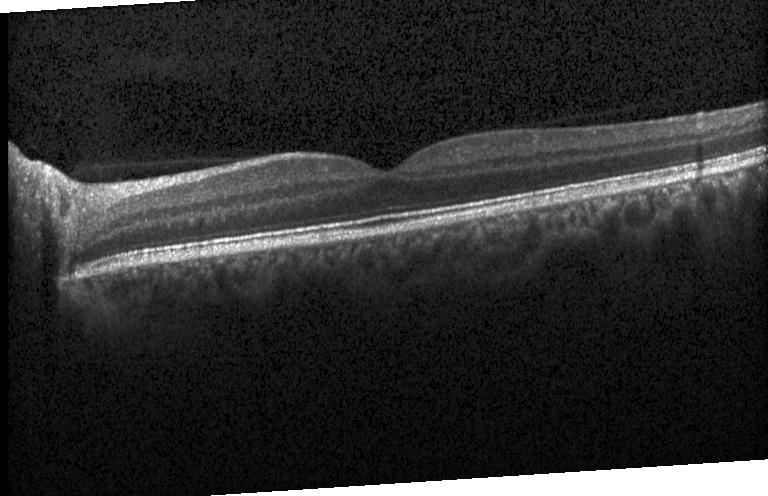
Macular OCT demonstrating no choroidal neovascularization, diabetic macular edema, or drusen.